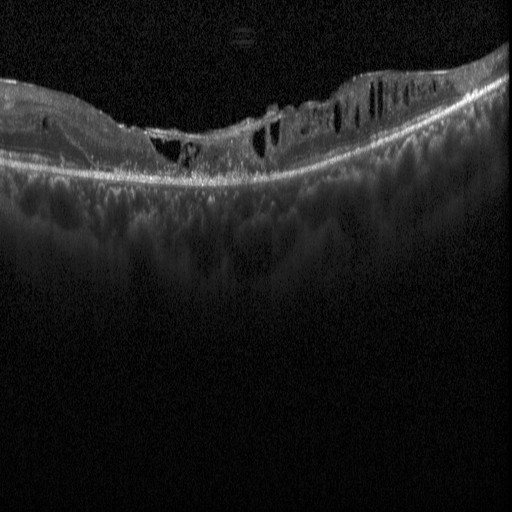
Spectral-domain optical coherence tomography; OCT B-scan. OCT finding: diabetic macular edema (DME).